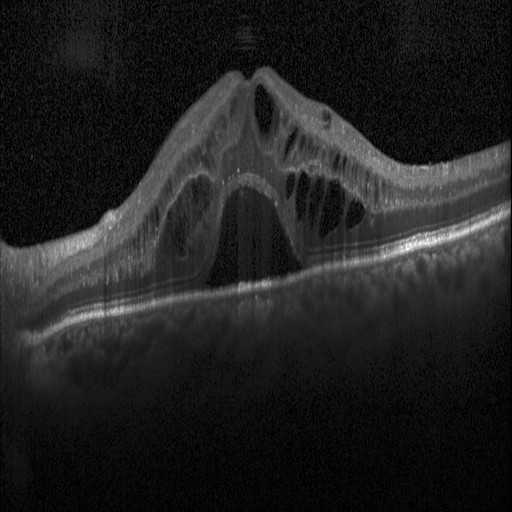
Spectral-domain optical coherence tomography; optical coherence tomography scan; through the macula
Impression: diabetic macular edema.